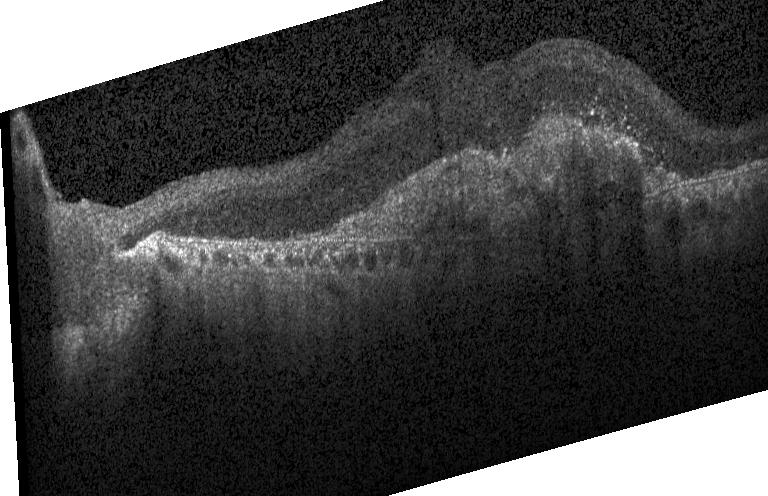
Diagnosis: choroidal neovascularization.